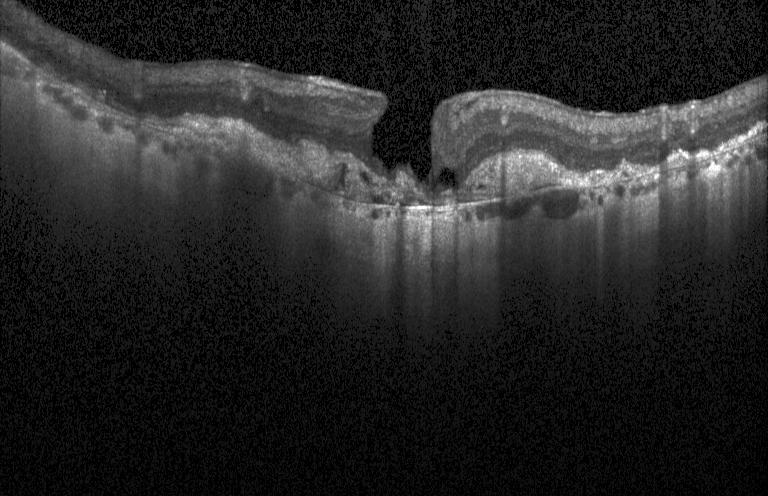 OCT finding: choroidal neovascularization.